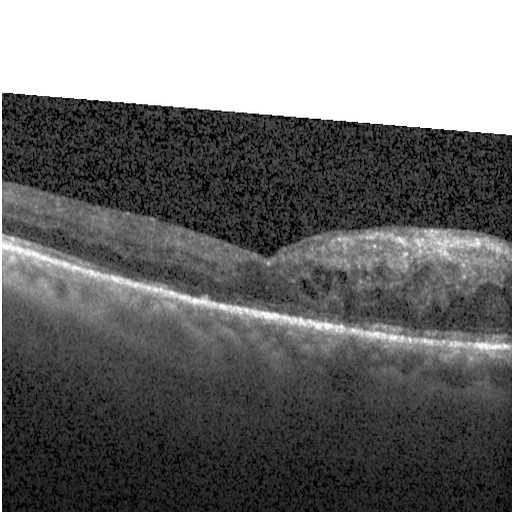

DME.